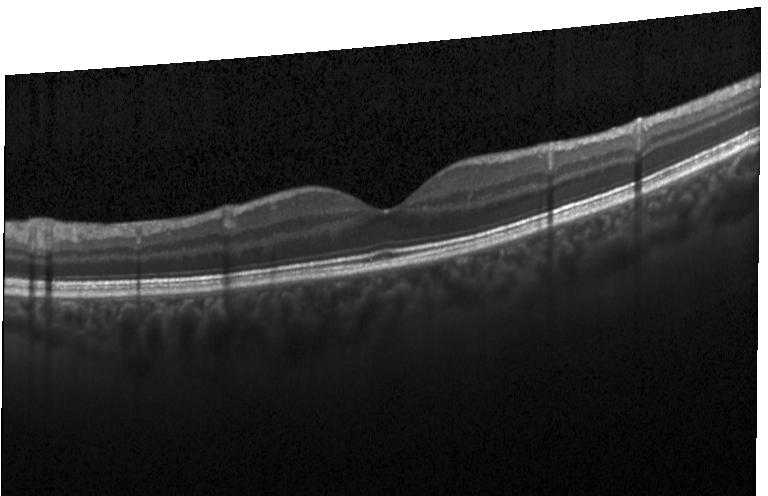 OCT B-scan showing neither choroidal neovascularization, diabetic macular edema, nor drusen.